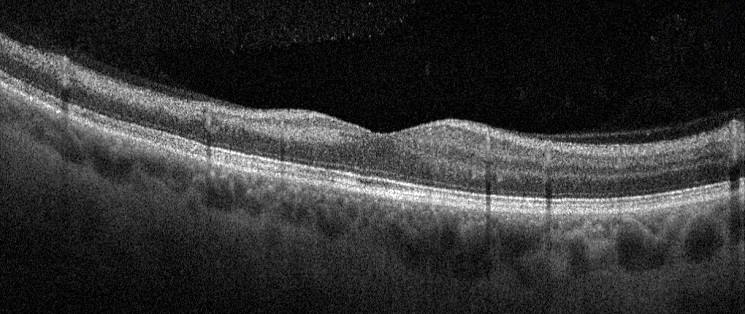 OCT line scan, through the macula. Diagnosis: retinal vein occlusion (RVO).